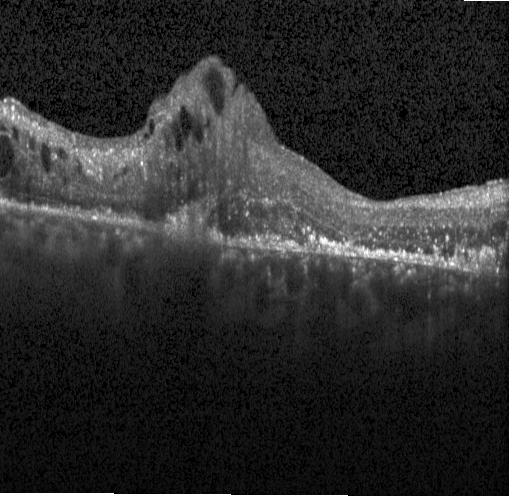 Optical coherence tomography B-scan. Diagnosis: choroidal neovascularization (CNV).